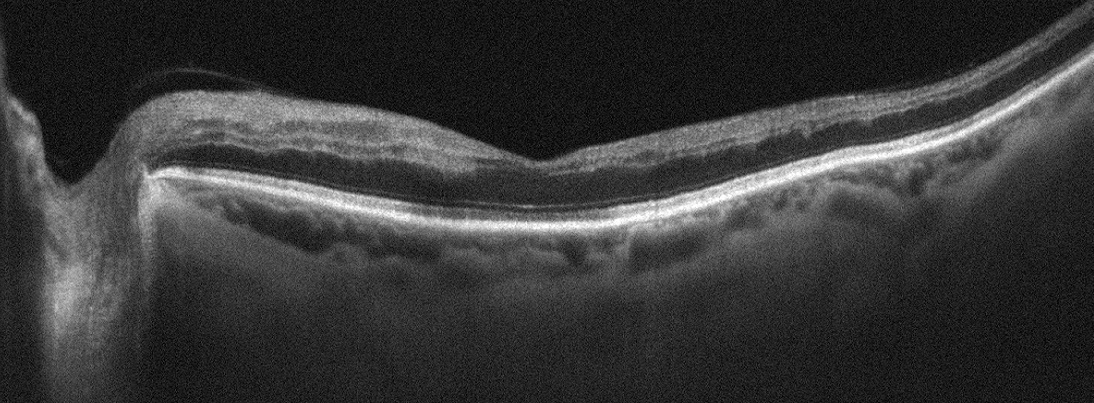 Instrument: Optovue Avanti RTVue XR · through the macula · retinal OCT cross-section
Finding: retinal vein occlusion.